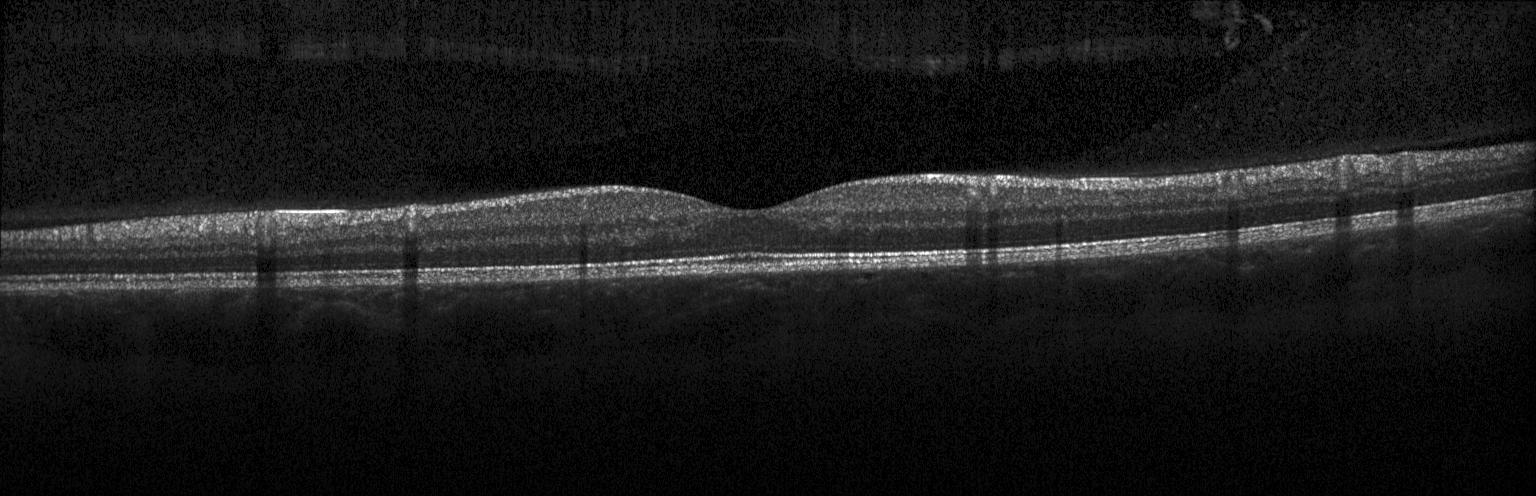

Macular scan; optical coherence tomography B-scan; Heidelberg Spectralis.
Finding: no CNV, DME, or drusen.